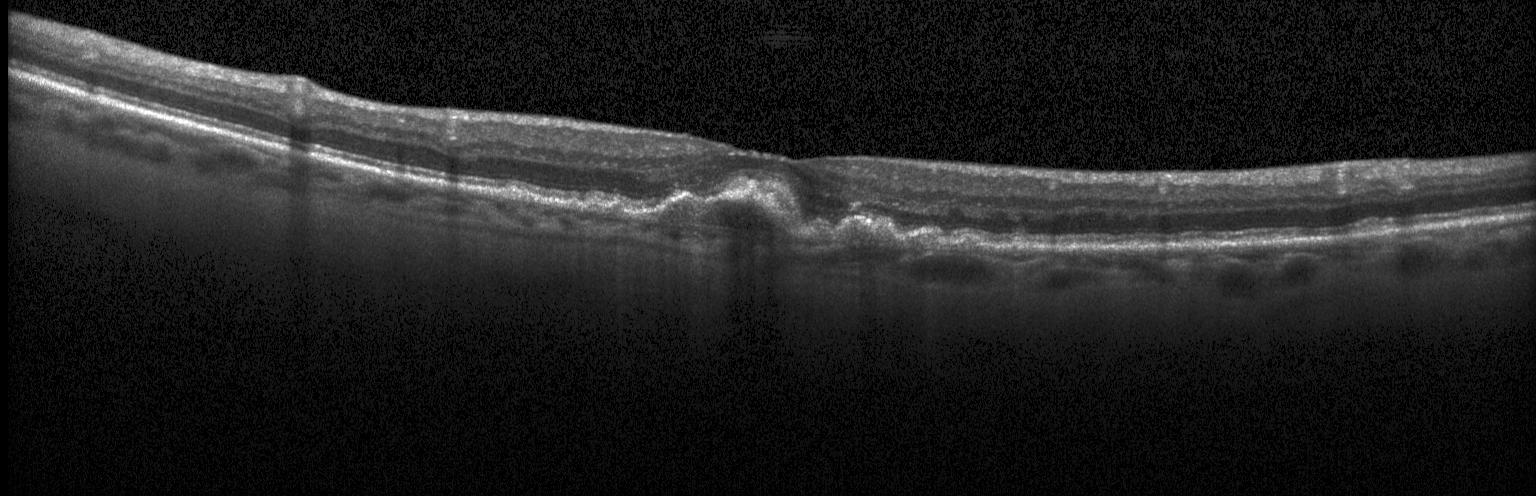

OCT line scan; spectral-domain optical coherence tomography; Heidelberg Spectralis OCT system — Impression: CNV.